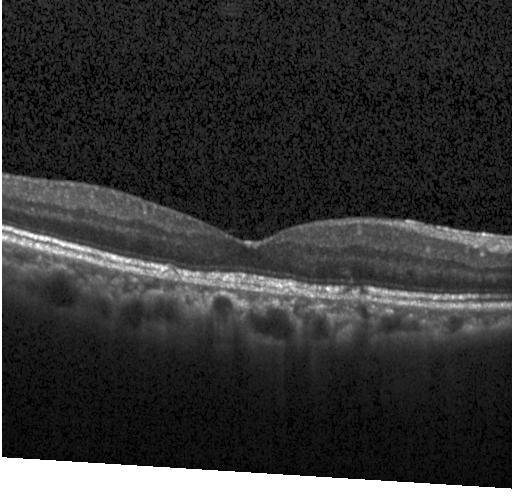 Impression: neither choroidal neovascularization, diabetic macular edema, nor drusen.